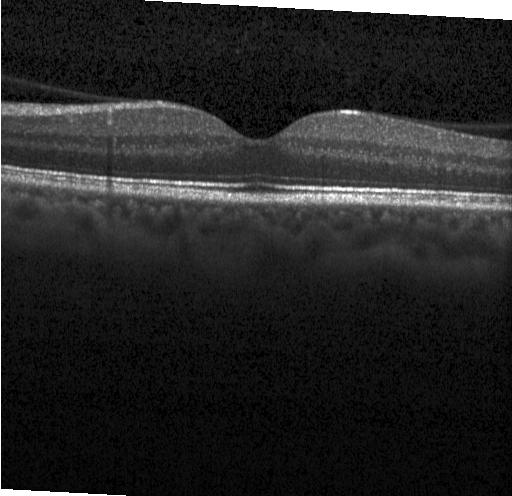 Assessment: no evidence of CNV, DME, or drusen.